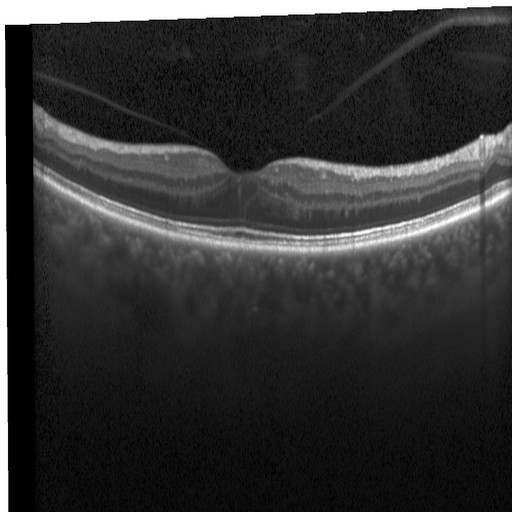

Impression: diabetic macular edema (DME).